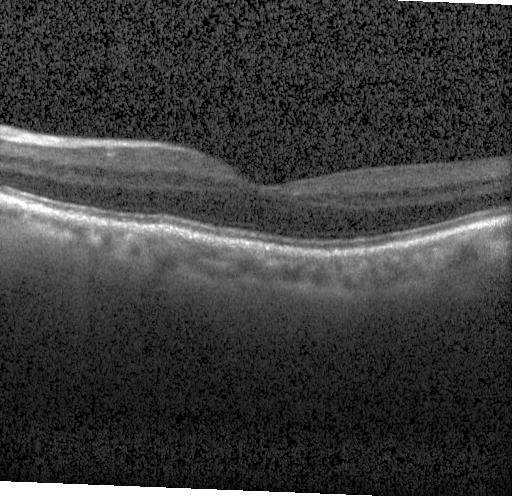

Dx: no choroidal neovascularization, diabetic macular edema, or drusen.